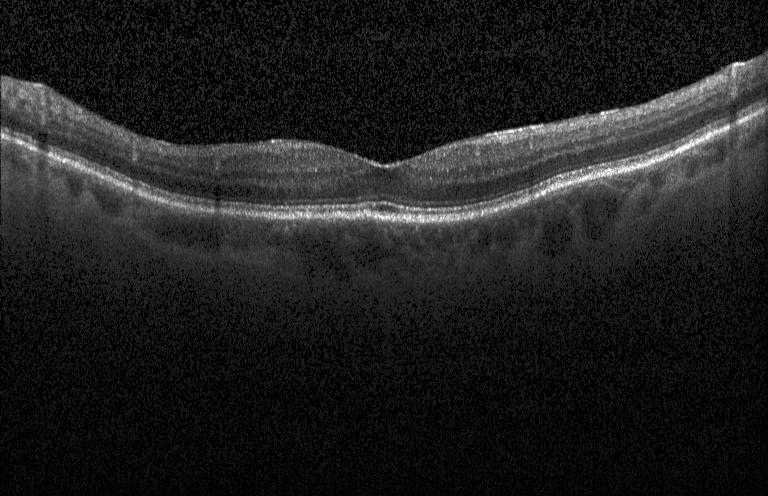 Impression: no CNV, DME, or drusen.